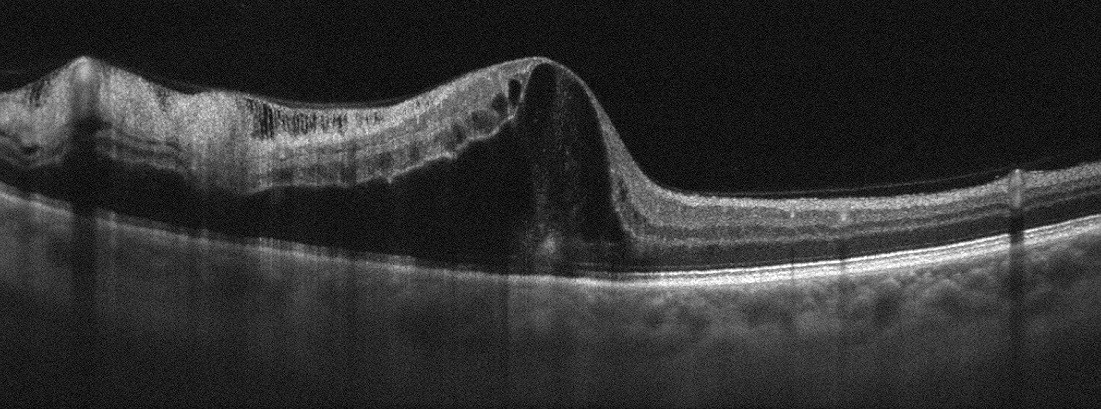
The scan shows RVO.